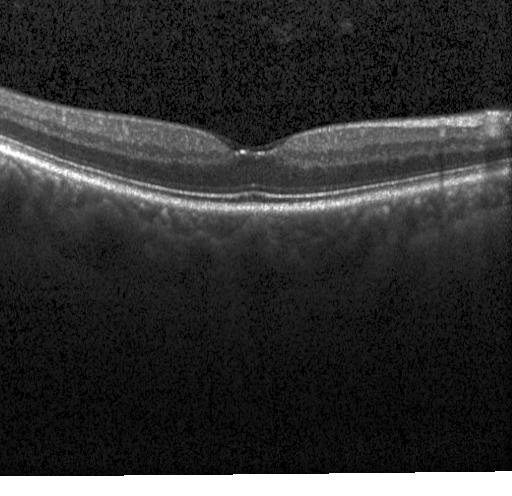

Instrument: Heidelberg Spectralis, optical coherence tomography B-scan, SD-OCT, horizontal scan through the fovea. OCT finding: neither choroidal neovascularization, diabetic macular edema, nor drusen.